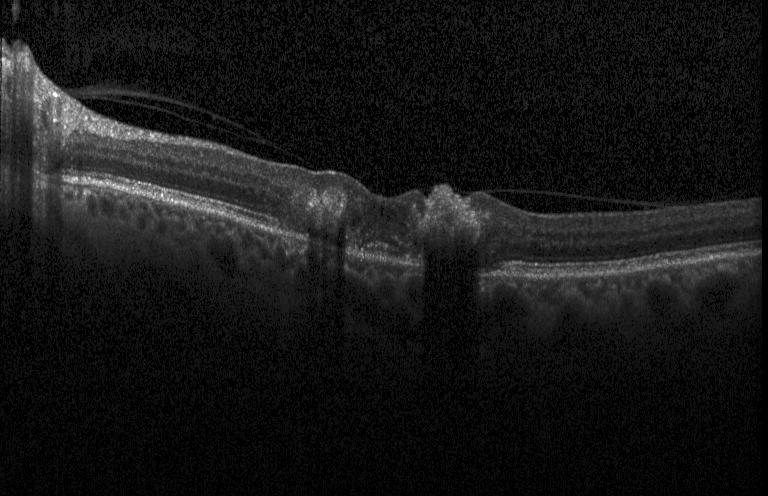
Retinal OCT B-scan; horizontal scan through the fovea. Impression: a choroidal neovascular membrane.